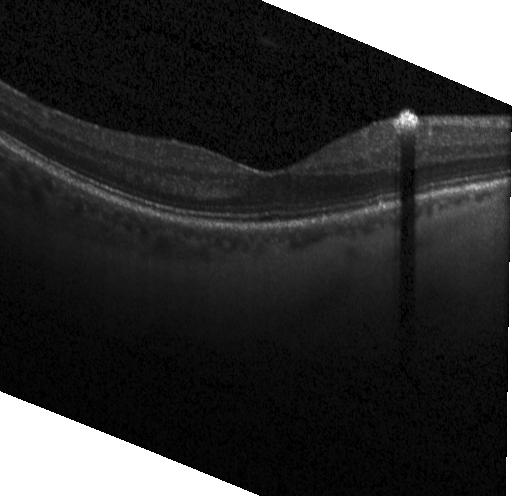
Optical coherence tomography B-scan; instrument: Heidelberg Spectralis; SD-OCT
The scan shows neither CNV, DME, nor drusen.